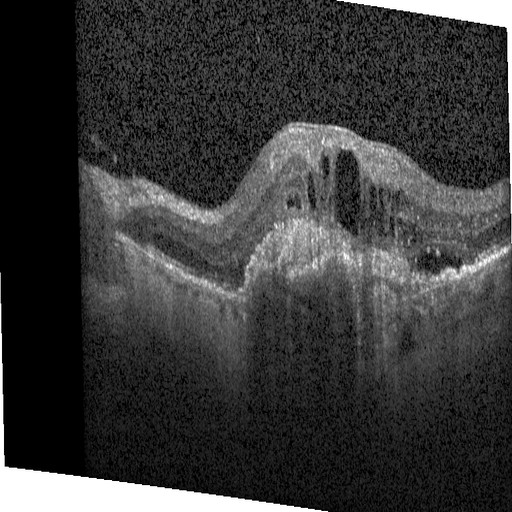

Spectral-domain optical coherence tomography. Optical coherence tomography scan
Impression: diabetic macular edema (DME).